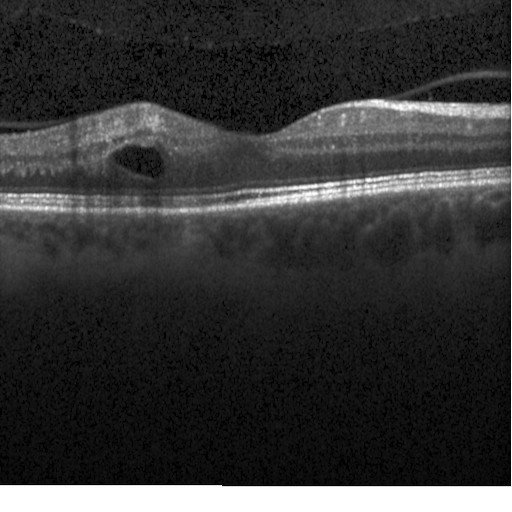

Retinal OCT B-scan. Impression: diabetic macular edema.